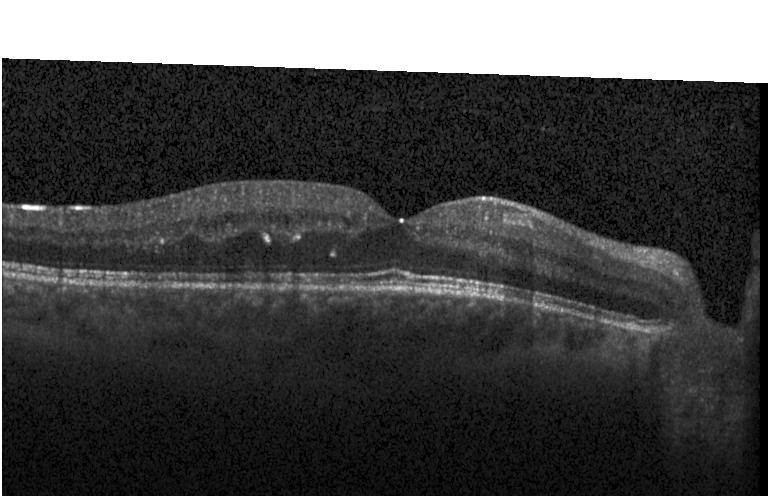
OCT finding: diabetic macular edema.